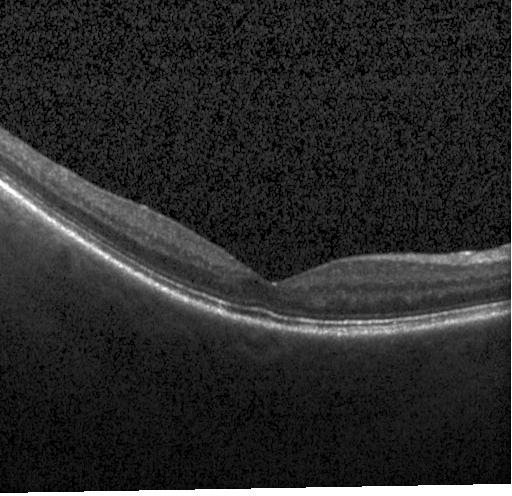

Macular OCT demonstrating no evidence of choroidal neovascularization, diabetic macular edema, or drusen.